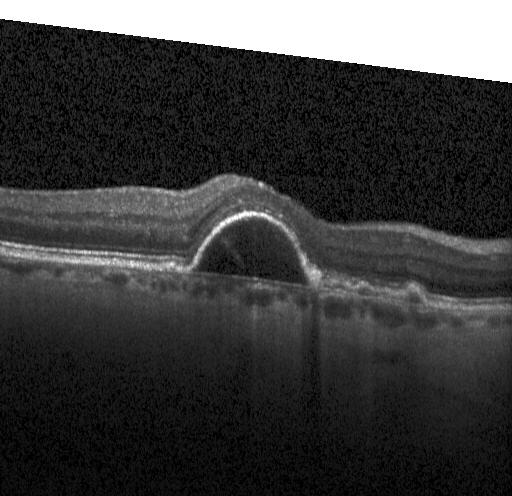
OCT line scan, horizontal scan through the fovea, SD-OCT, instrument: Heidelberg Spectralis
Impression: a choroidal neovascular membrane.